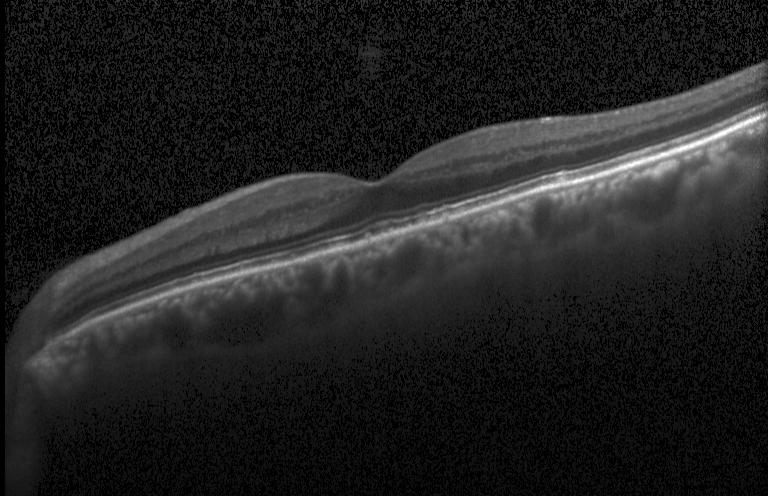
Finding: multiple drusen.